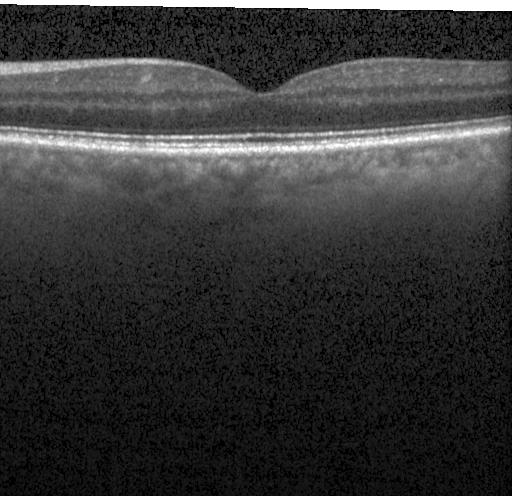

This B-scan demonstrates no CNV, no DME, and no drusen.